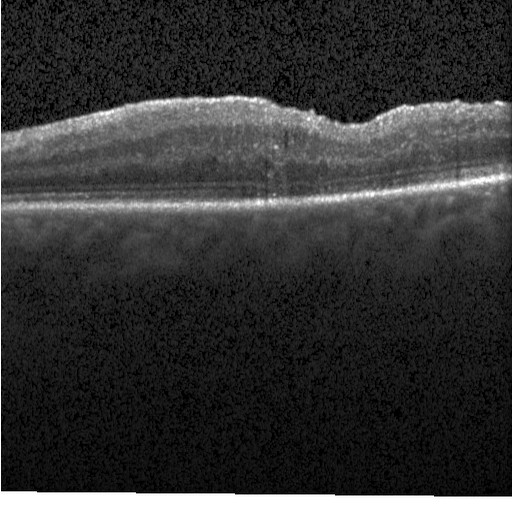
Retinal OCT cross-section showing diabetic macular edema.